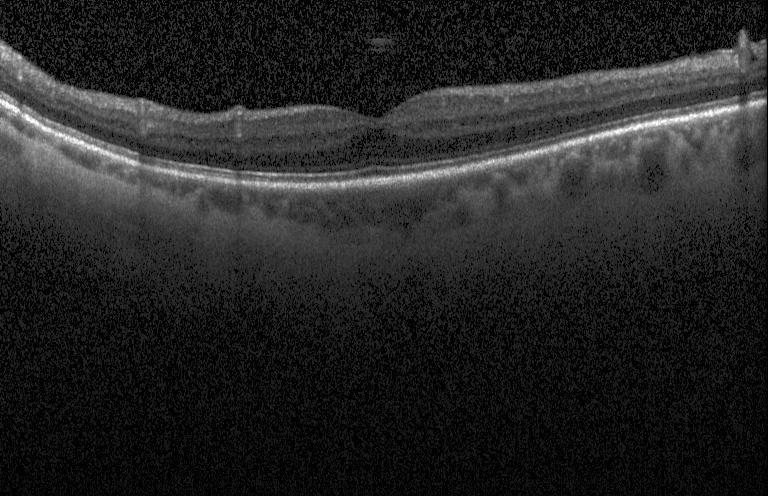 Optical coherence tomography scan. Centered on the fovea. SD-OCT — Assessment: neither choroidal neovascularization, diabetic macular edema, nor drusen.